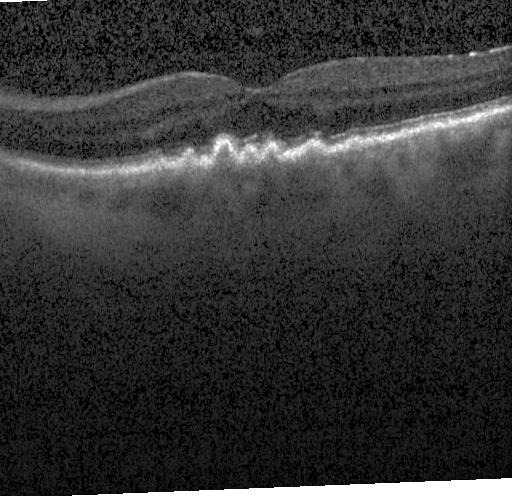

Impression: sub-RPE drusenoid deposits.